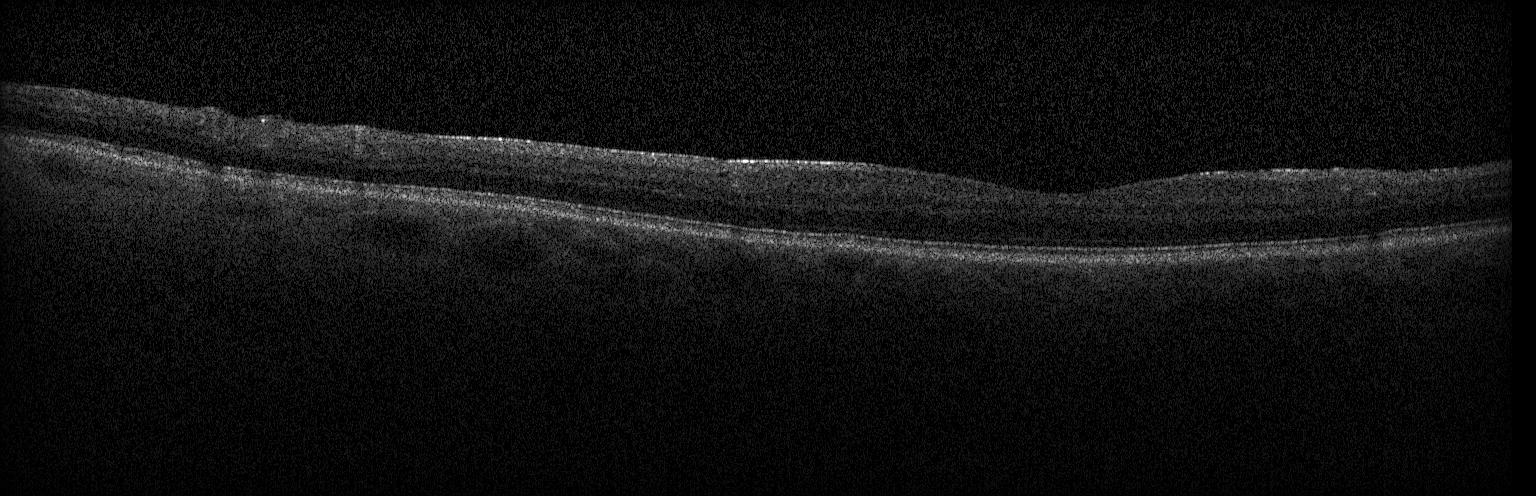 Instrument: Heidelberg Spectralis; optical coherence tomography scan — OCT finding: no evidence of CNV, DME, or drusen.